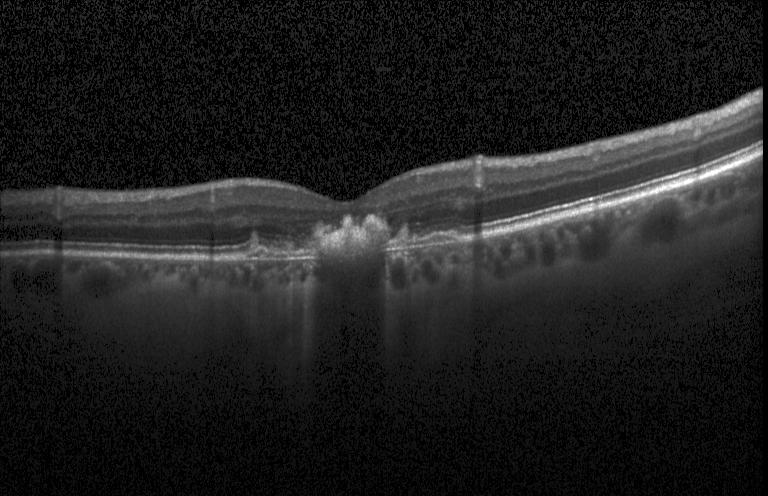

Optical coherence tomography scan. OCT finding: a choroidal neovascular membrane.